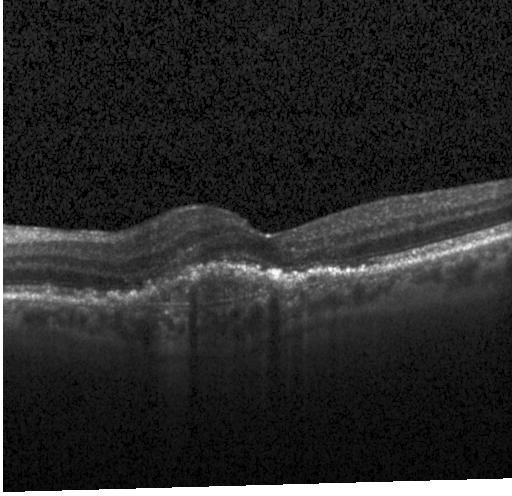 Acquired on a Heidelberg Spectralis, optical coherence tomography scan, spectral-domain optical coherence tomography. OCT finding: CNV.